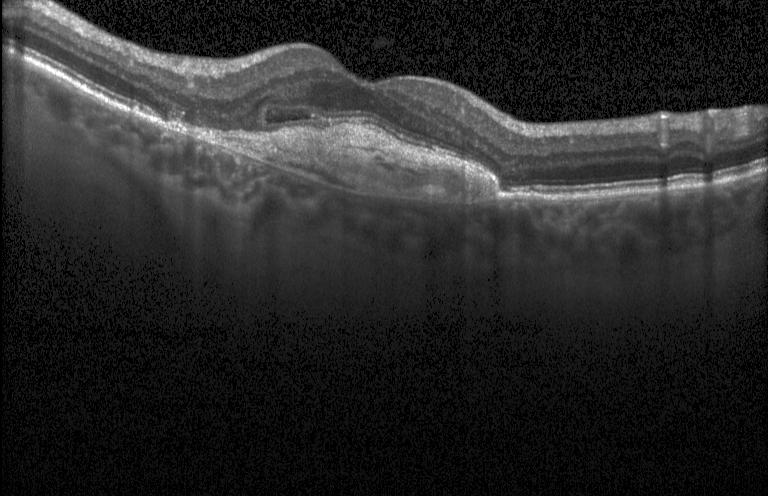 Macular OCT demonstrating CNV.